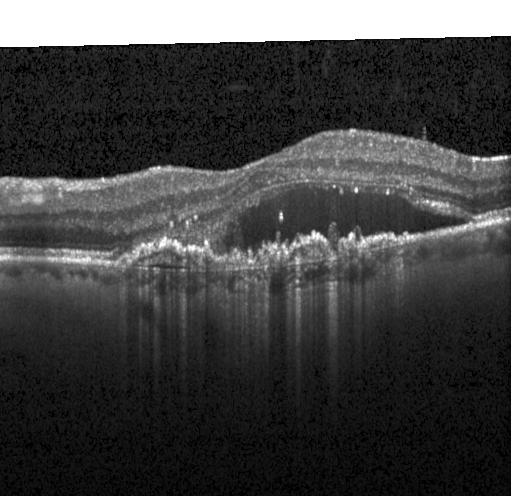 Assessment: a choroidal neovascular membrane.